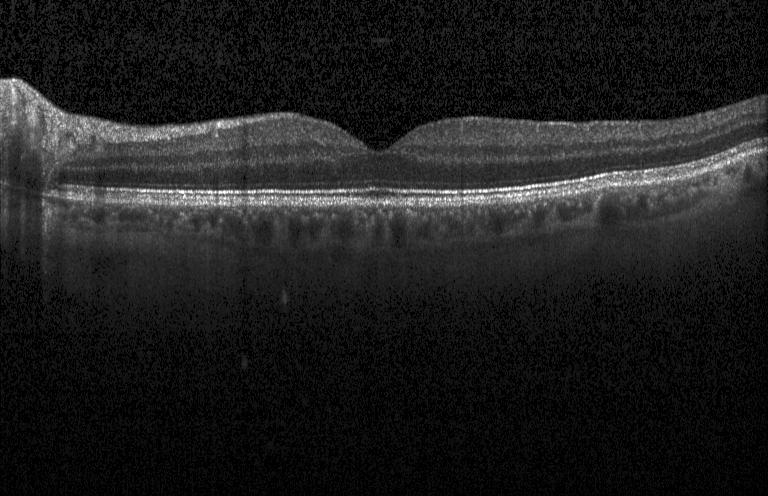

Macular scan; optical coherence tomography scan — Dx: neither choroidal neovascularization, diabetic macular edema, nor drusen.